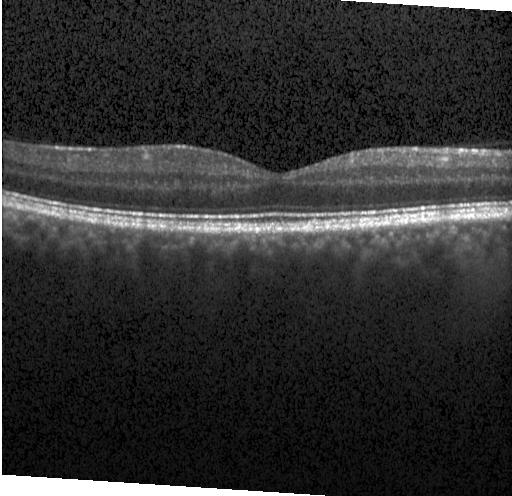 Finding: no evidence of CNV, DME, or drusen.